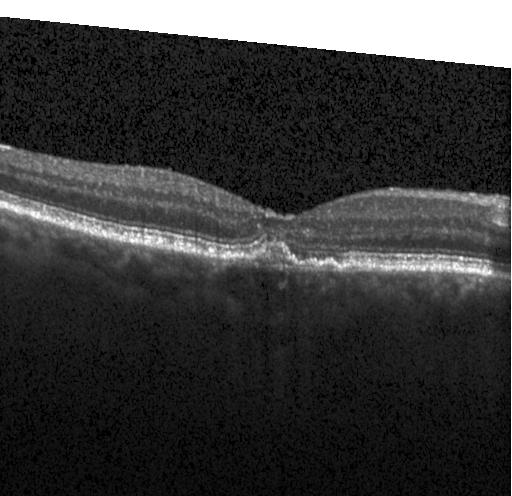

OCT scan showing sub-RPE drusenoid deposits.